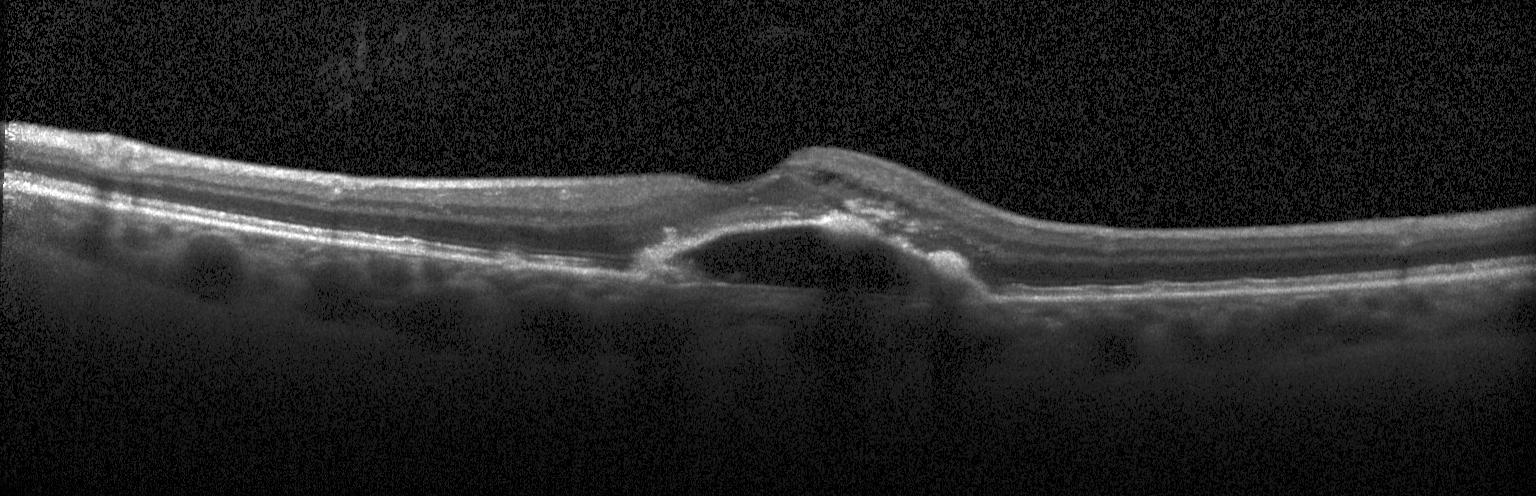 SD-OCT · acquired on a Heidelberg Spectralis · horizontal scan through the fovea · retinal OCT cross-section. Choroidal neovascularization.